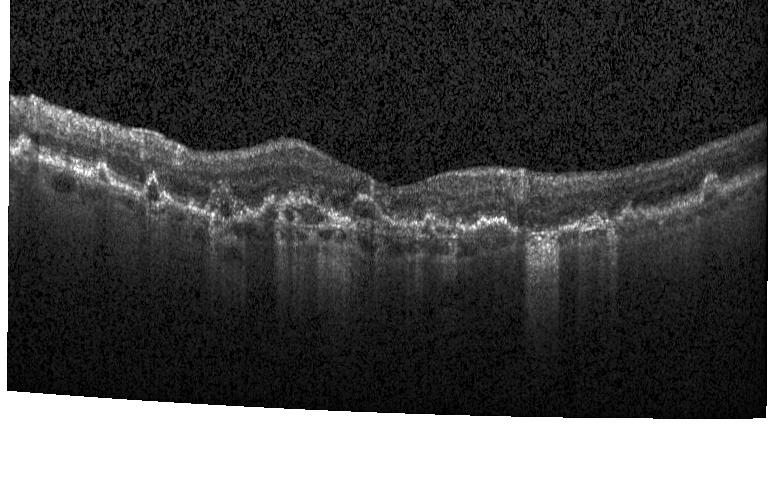

SD-OCT. Retinal OCT cross-section. Horizontal scan through the fovea.
This B-scan demonstrates a choroidal neovascular membrane.